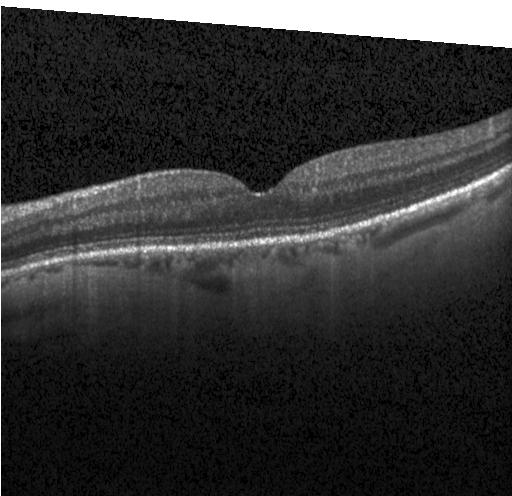
Optical coherence tomography scan; centered on the fovea; Heidelberg Spectralis. Finding: no evidence of choroidal neovascularization, diabetic macular edema, or drusen.